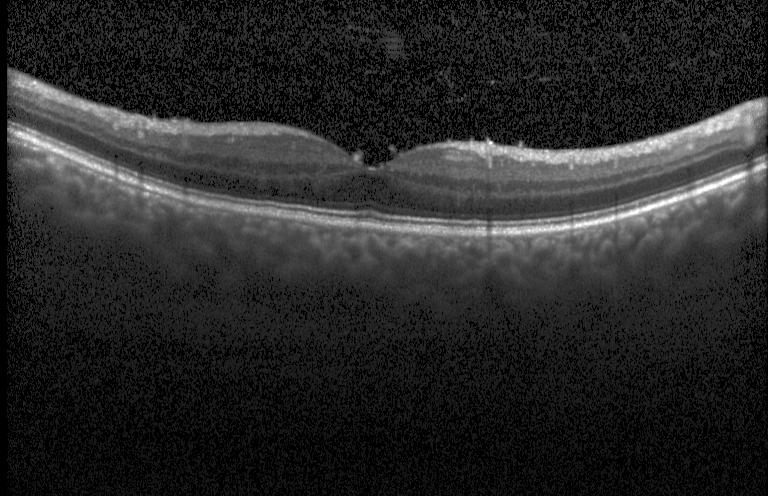
Macular OCT: no choroidal neovascularization, diabetic macular edema, or drusen.